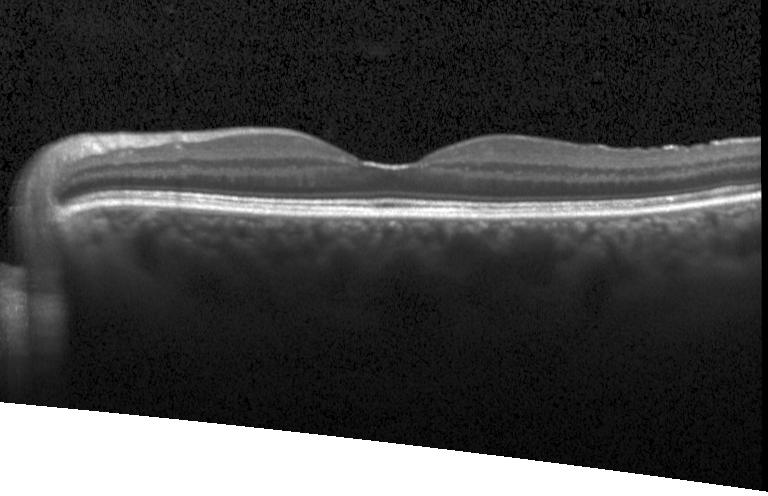 Retinal OCT B-scan; fovea-centered. Assessment: no choroidal neovascularization, diabetic macular edema, or drusen.